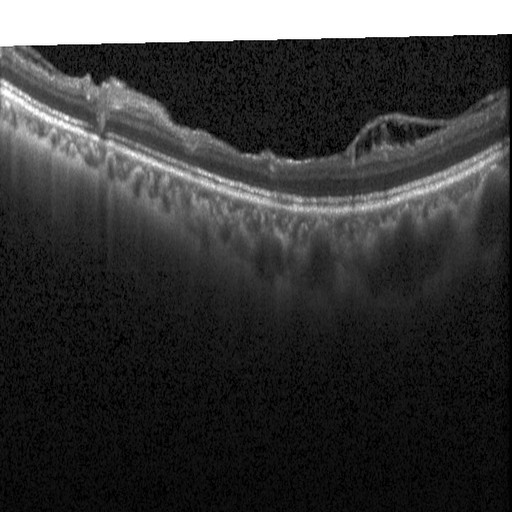

Finding: diabetic macular edema.